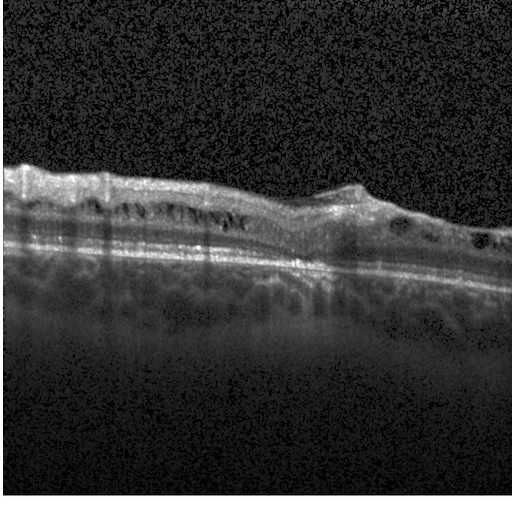
Macular OCT: diabetic macular edema.